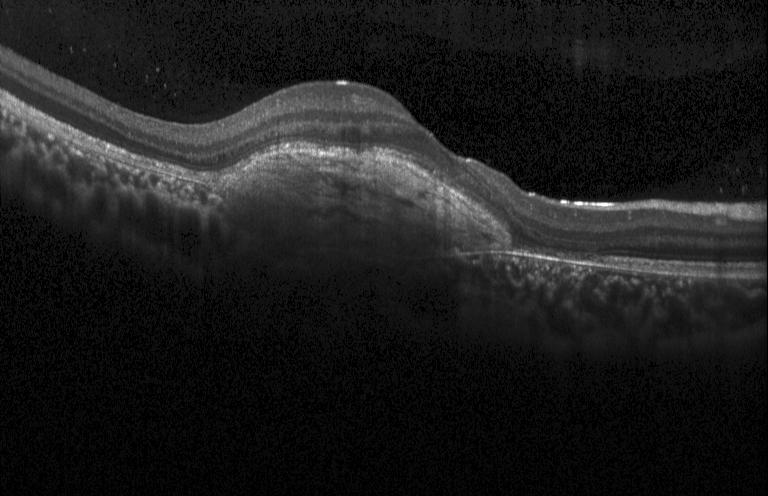
Dx: a choroidal neovascular membrane.